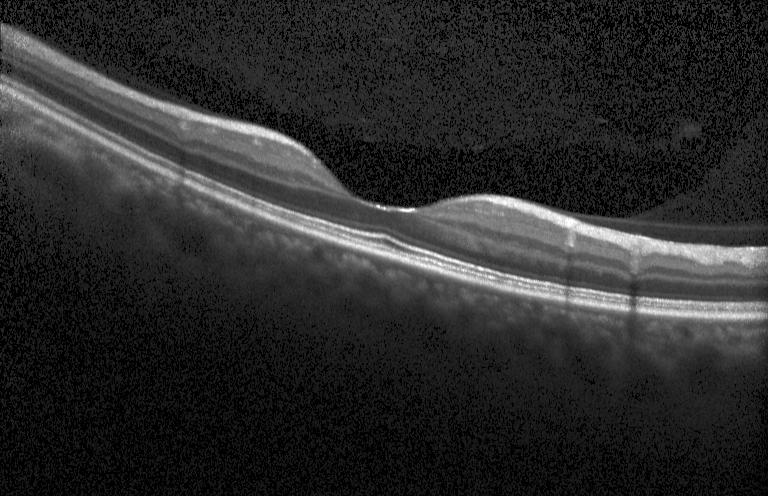
Fovea-centered; retinal OCT B-scan. This B-scan demonstrates no CNV, DME, or drusen.